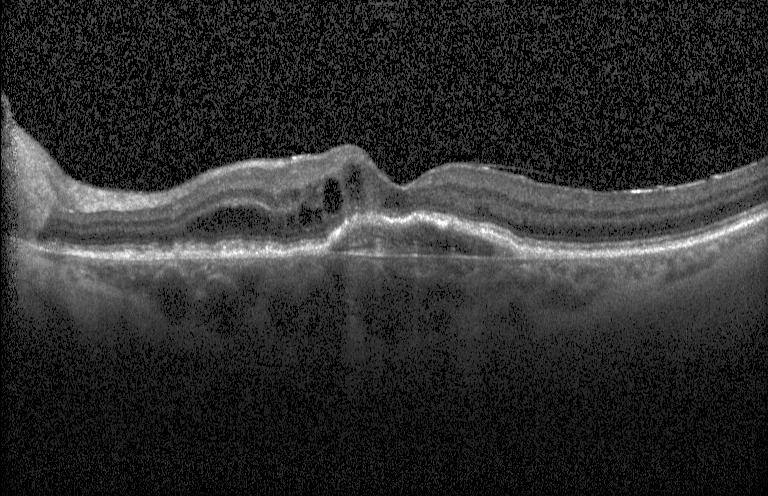

Centered on the fovea; Heidelberg Spectralis OCT system; retinal OCT B-scan. Dx: choroidal neovascularization (CNV).